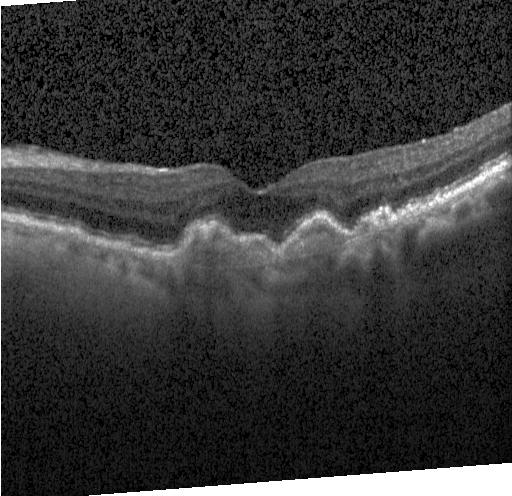 Through the macula, OCT B-scan.
Finding: a choroidal neovascular membrane.